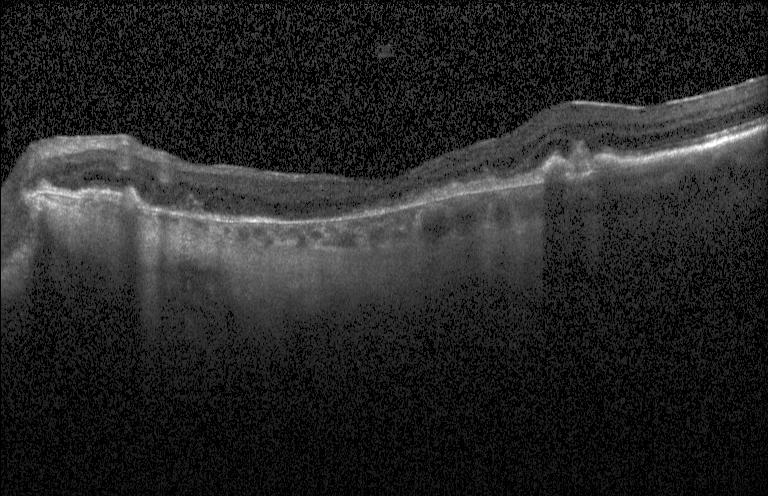 Spectral-domain OCT B-scan: a choroidal neovascular membrane.